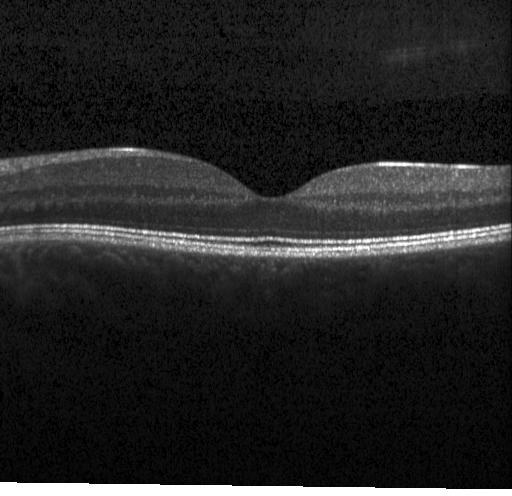 Spectral-domain OCT, retinal OCT cross-section — OCT finding: no evidence of choroidal neovascularization, diabetic macular edema, or drusen.